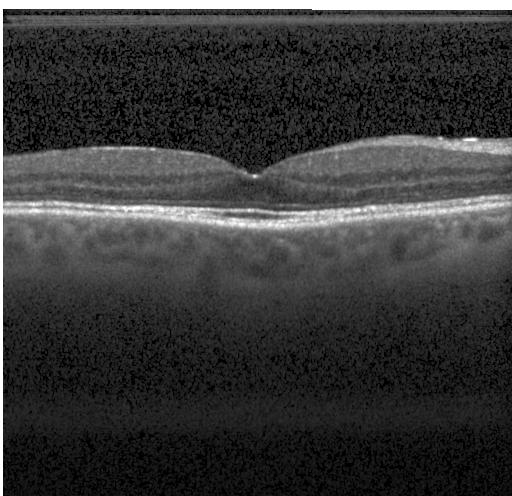
Optical coherence tomography scan; horizontal scan through the fovea; SD-OCT — Assessment: neither CNV, DME, nor drusen.